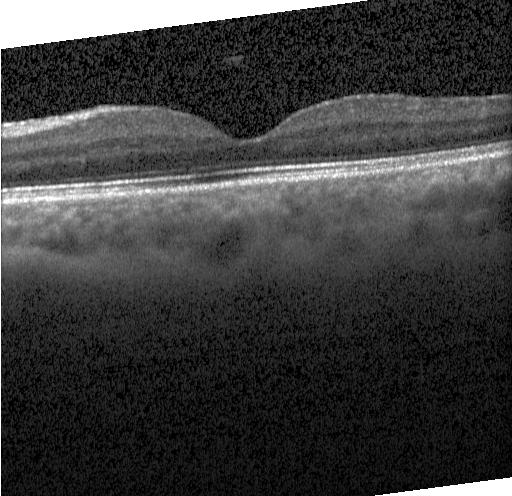

Heidelberg Spectralis OCT system; OCT line scan. Finding: neither CNV, DME, nor drusen.